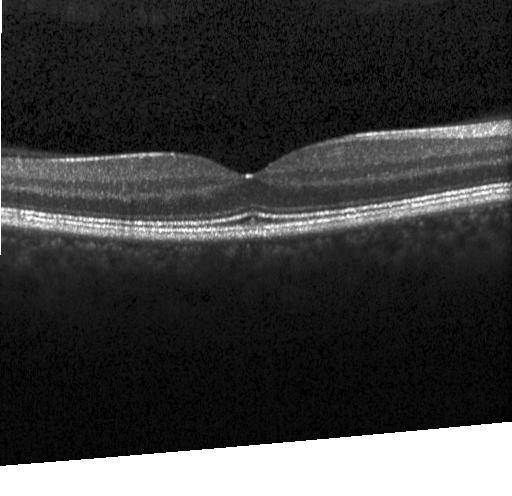 Impression: neither choroidal neovascularization, diabetic macular edema, nor drusen.